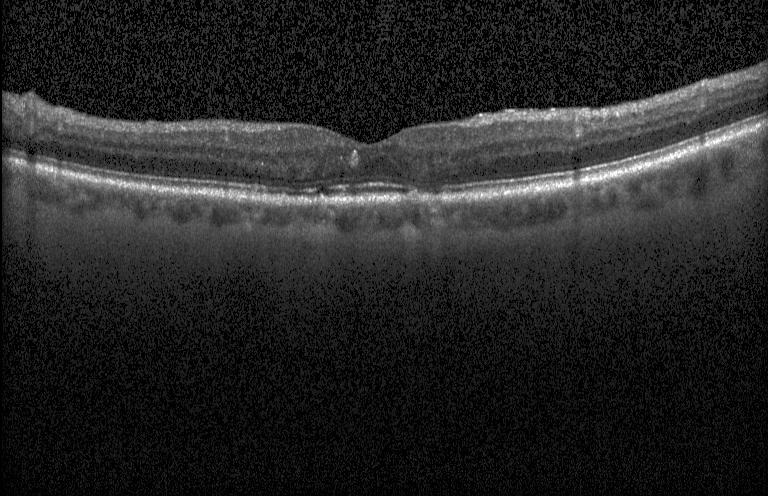

This B-scan demonstrates diabetic macular edema.